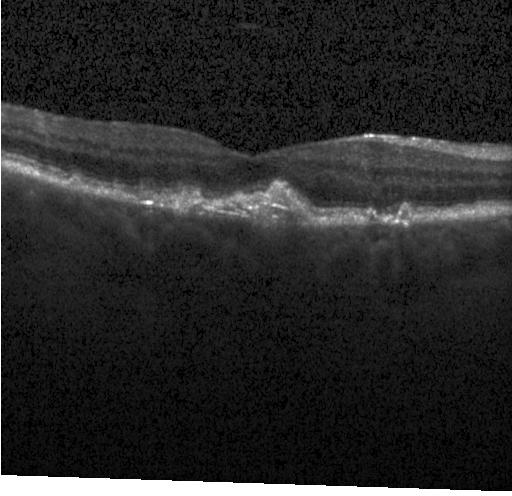
OCT B-scan showing a choroidal neovascular membrane.